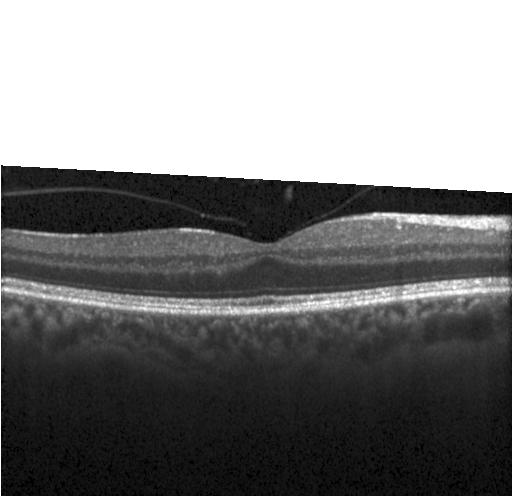

OCT B-scan showing no choroidal neovascularization, diabetic macular edema, or drusen.